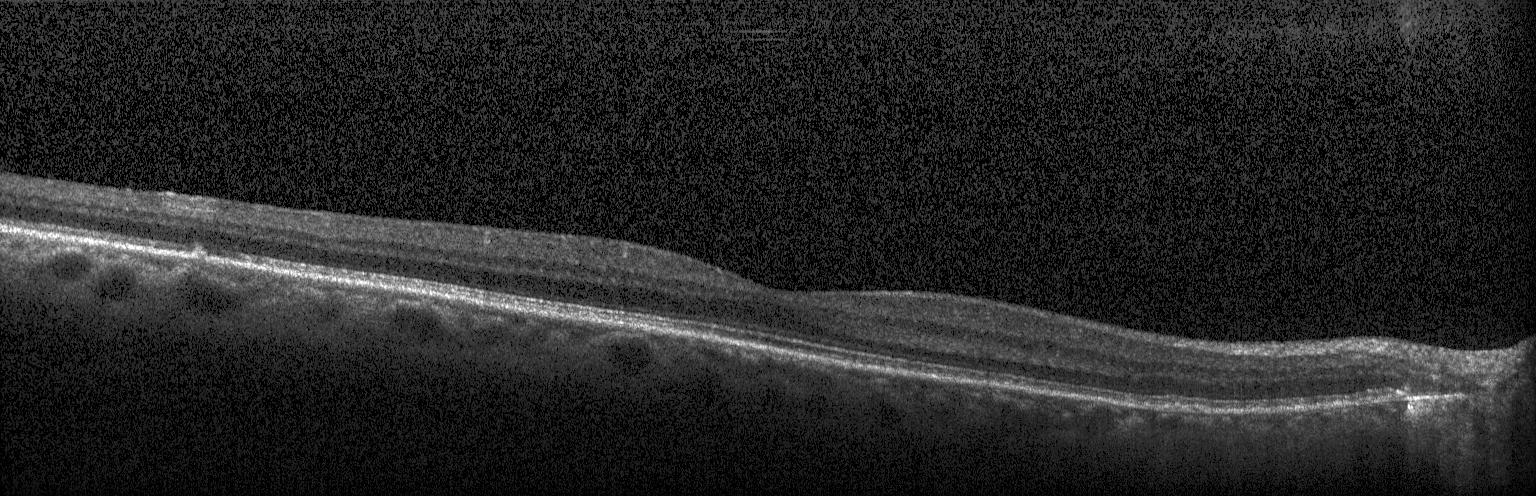 Retinal OCT cross-section
Macular OCT: neither choroidal neovascularization, diabetic macular edema, nor drusen.